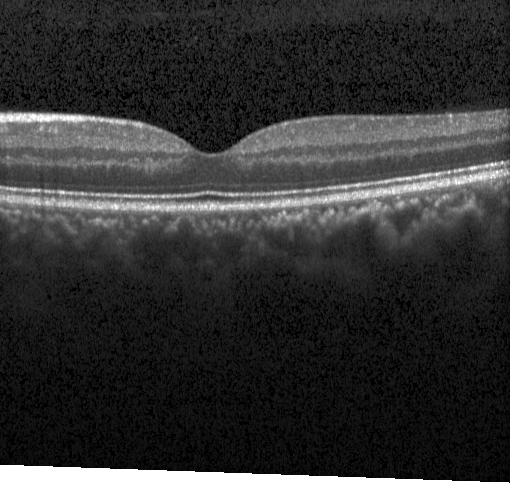

OCT finding: no choroidal neovascularization, diabetic macular edema, or drusen.